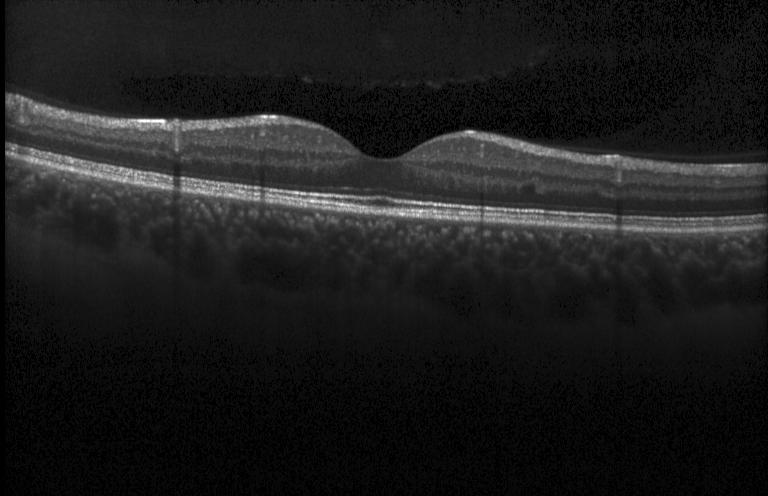

Macular OCT demonstrating neither CNV, DME, nor drusen.